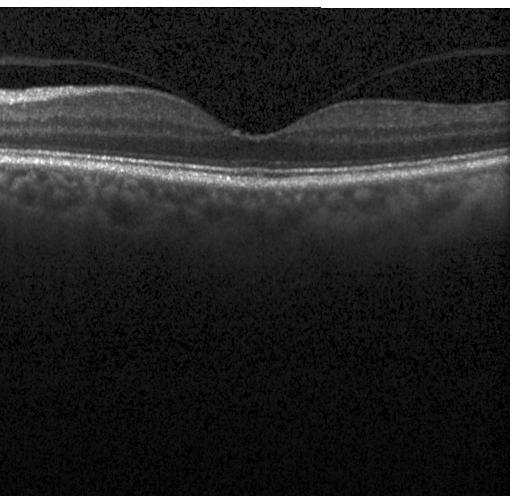

OCT line scan. Fovea-centered. SD-OCT. Heidelberg Spectralis
Assessment: no evidence of choroidal neovascularization, diabetic macular edema, or drusen.